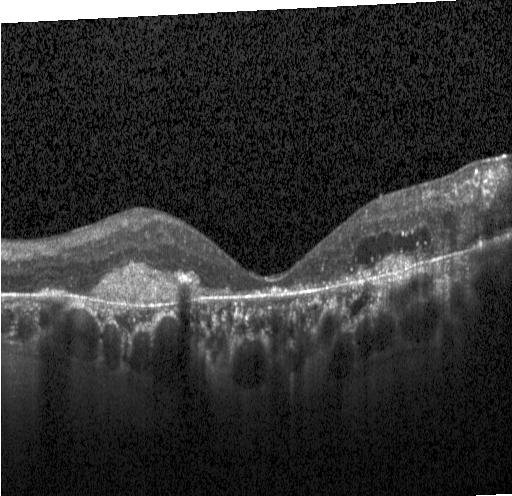 OCT scan showing choroidal neovascularization.